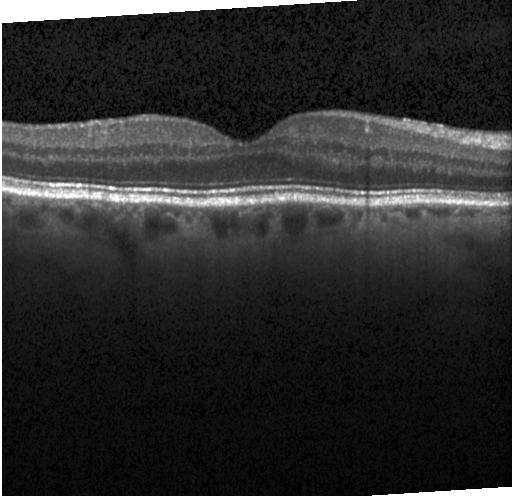

Retinal OCT B-scan — Finding: no choroidal neovascularization, diabetic macular edema, or drusen.